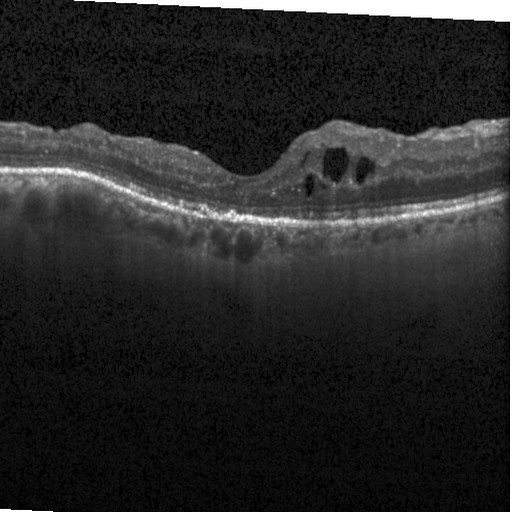 Retinal OCT cross-section; spectral-domain optical coherence tomography; Heidelberg Spectralis OCT system; centered on the fovea. Finding: diabetic macular edema.